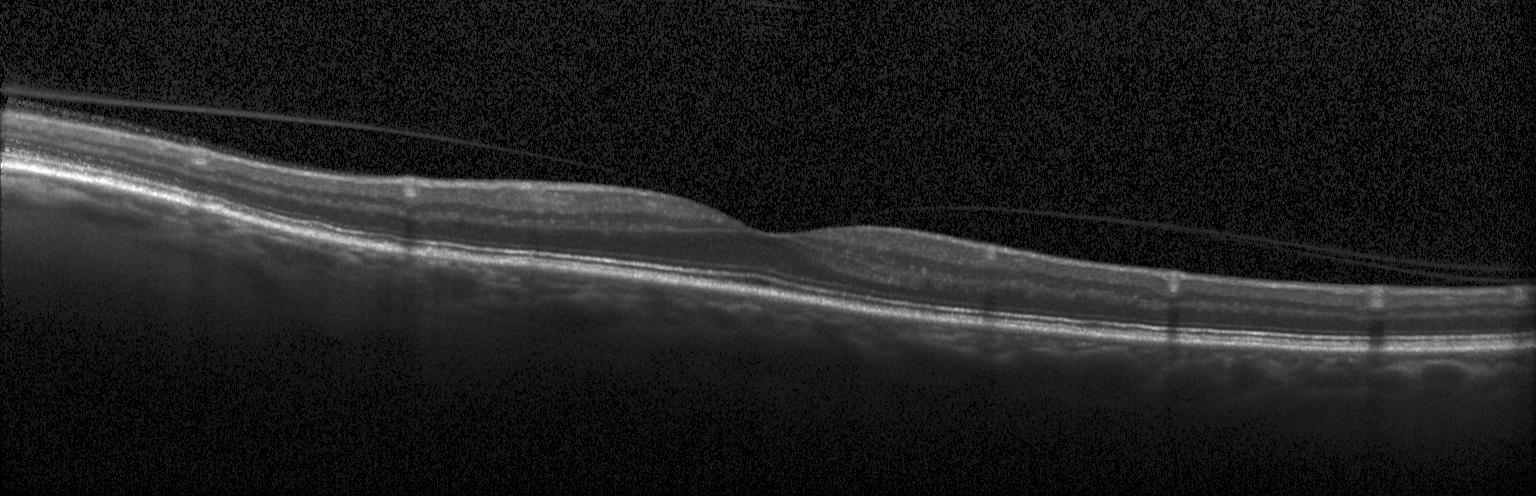 Optical coherence tomography scan, SD-OCT — Macular OCT: no evidence of choroidal neovascularization, diabetic macular edema, or drusen.